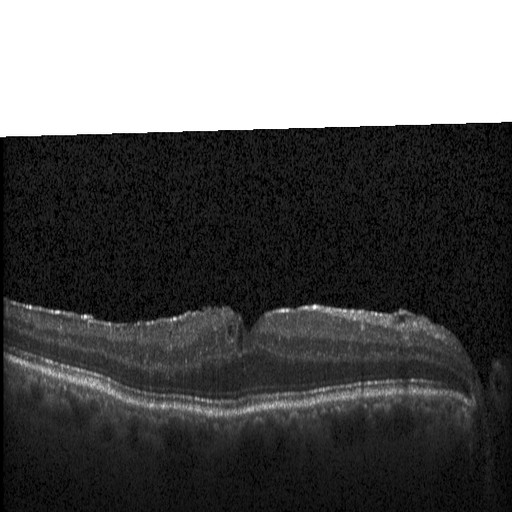 Horizontal scan through the fovea · instrument: Heidelberg Spectralis · optical coherence tomography scan · SD-OCT — Assessment: diabetic macular edema (DME).